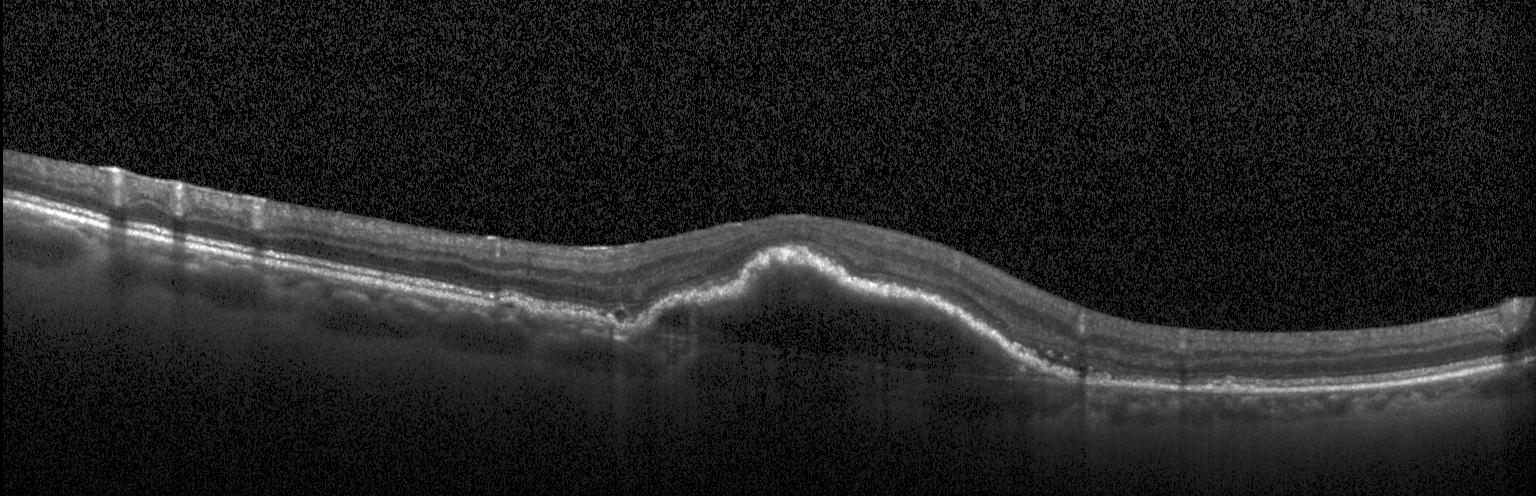
Spectral-domain OCT; optical coherence tomography scan; Heidelberg Spectralis OCT system — A choroidal neovascular membrane.